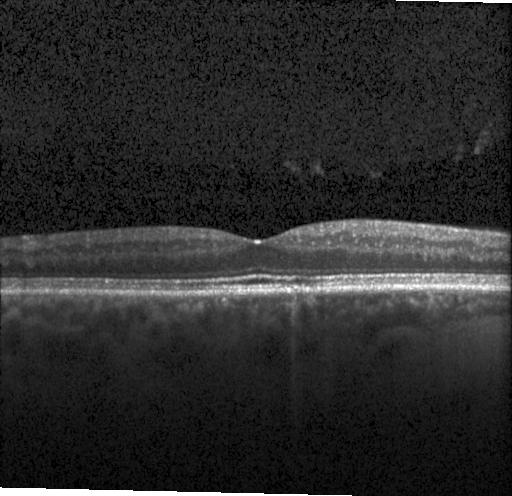

Heidelberg Spectralis. Optical coherence tomography scan. Macular scan. Spectral-domain OCT
Assessment: no CNV, DME, or drusen.